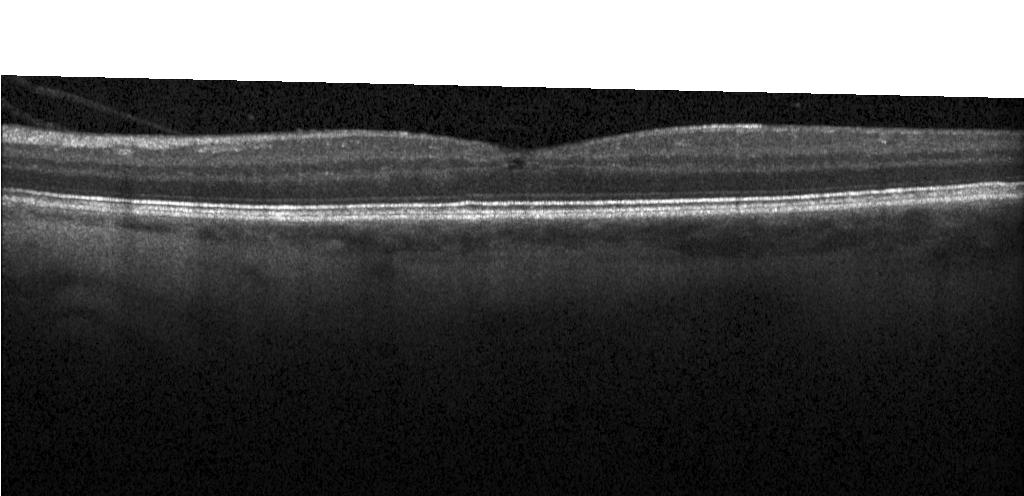

SD-OCT; Heidelberg Spectralis OCT system; optical coherence tomography scan. Assessment: neither choroidal neovascularization, diabetic macular edema, nor drusen.